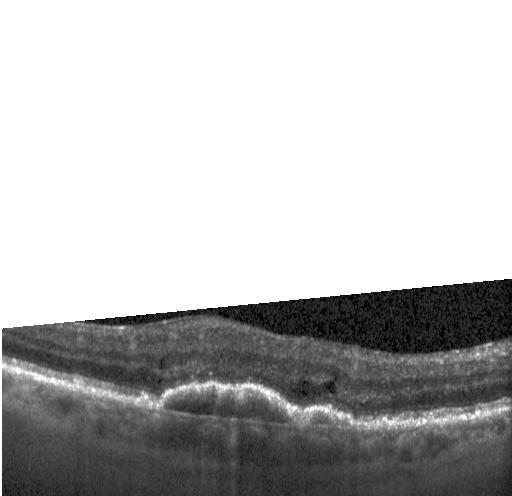 SD-OCT, Heidelberg Spectralis, OCT B-scan, horizontal scan through the fovea. Dx: CNV.